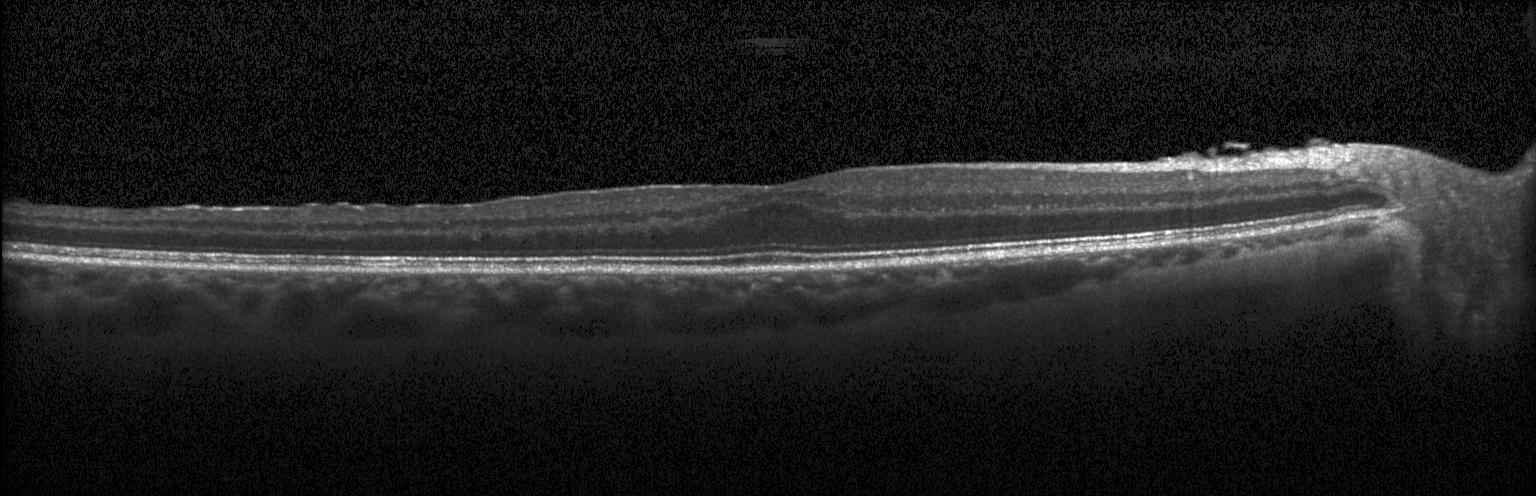 OCT B-scan — Finding: no evidence of CNV, DME, or drusen.